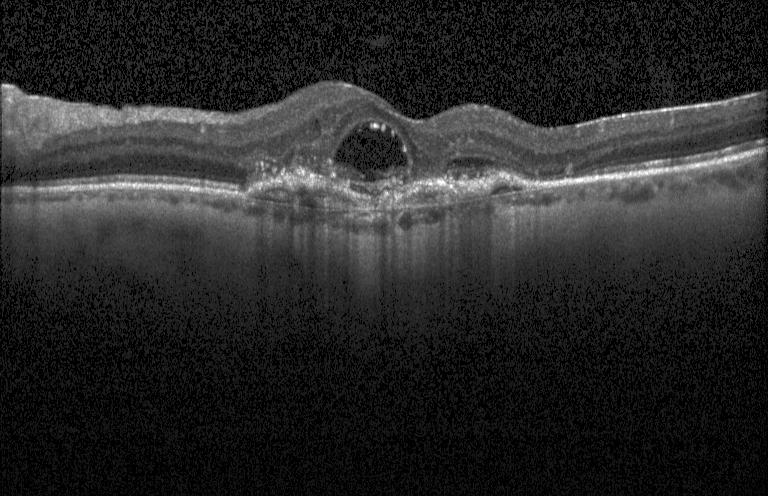 Spectral-domain optical coherence tomography, optical coherence tomography scan.
Impression: a choroidal neovascular membrane.